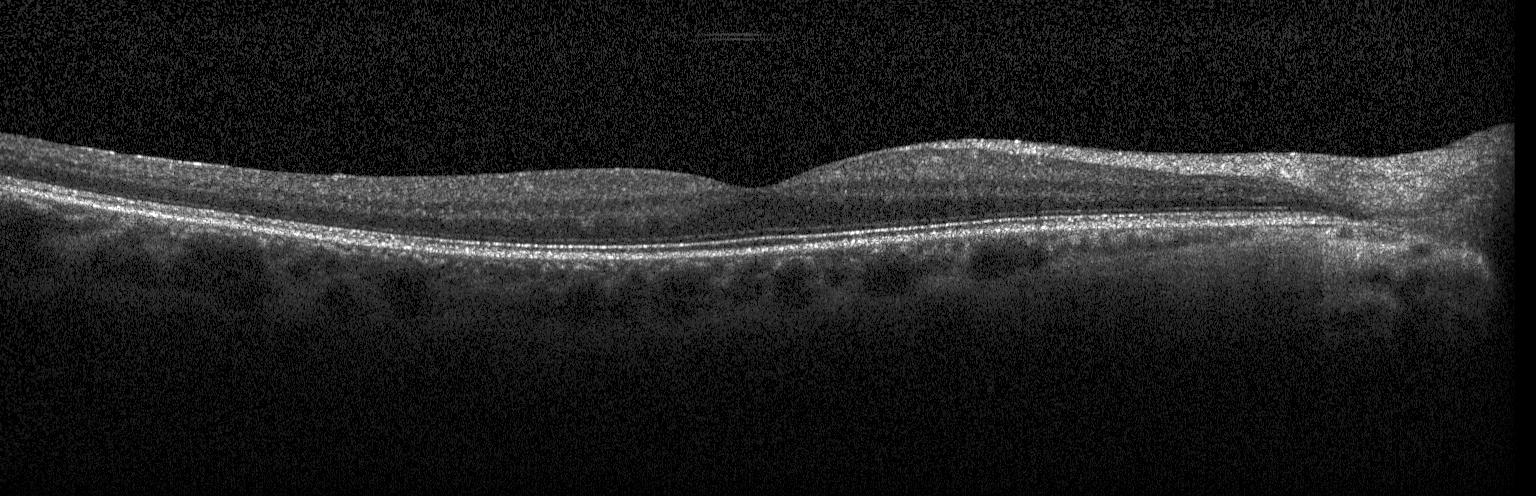 OCT B-scan, macular scan, instrument: Heidelberg Spectralis — Finding: no evidence of choroidal neovascularization, diabetic macular edema, or drusen.